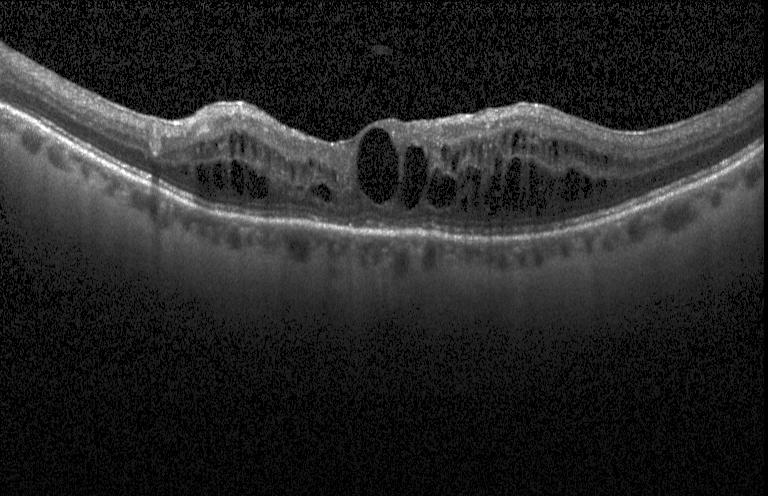

Spectral-domain OCT · OCT B-scan — Finding: DME.